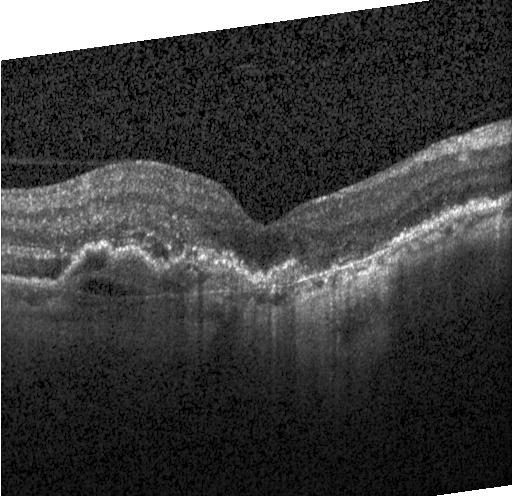

SD-OCT. Fovea-centered. OCT B-scan
A choroidal neovascular membrane.